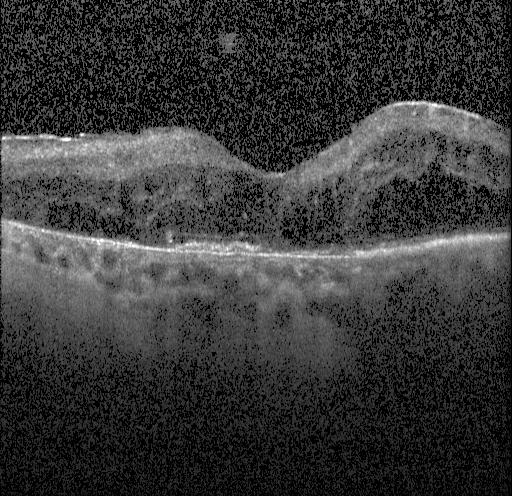 Horizontal scan through the fovea. OCT B-scan. Heidelberg Spectralis
Assessment: a choroidal neovascular membrane.